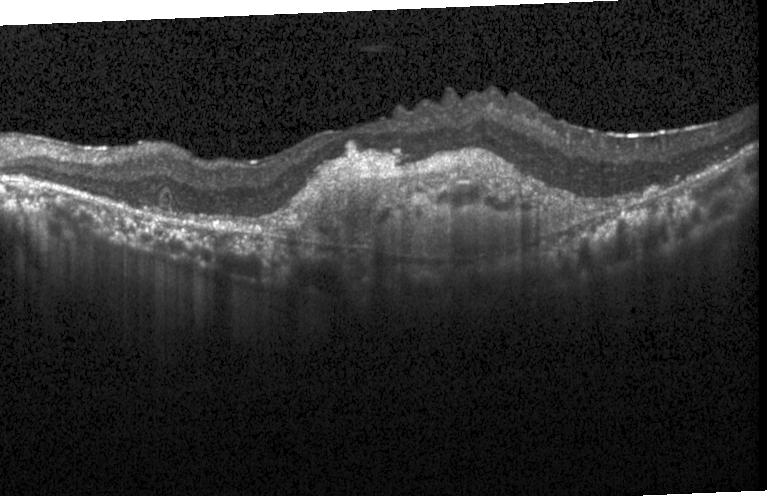

Finding: a choroidal neovascular membrane.